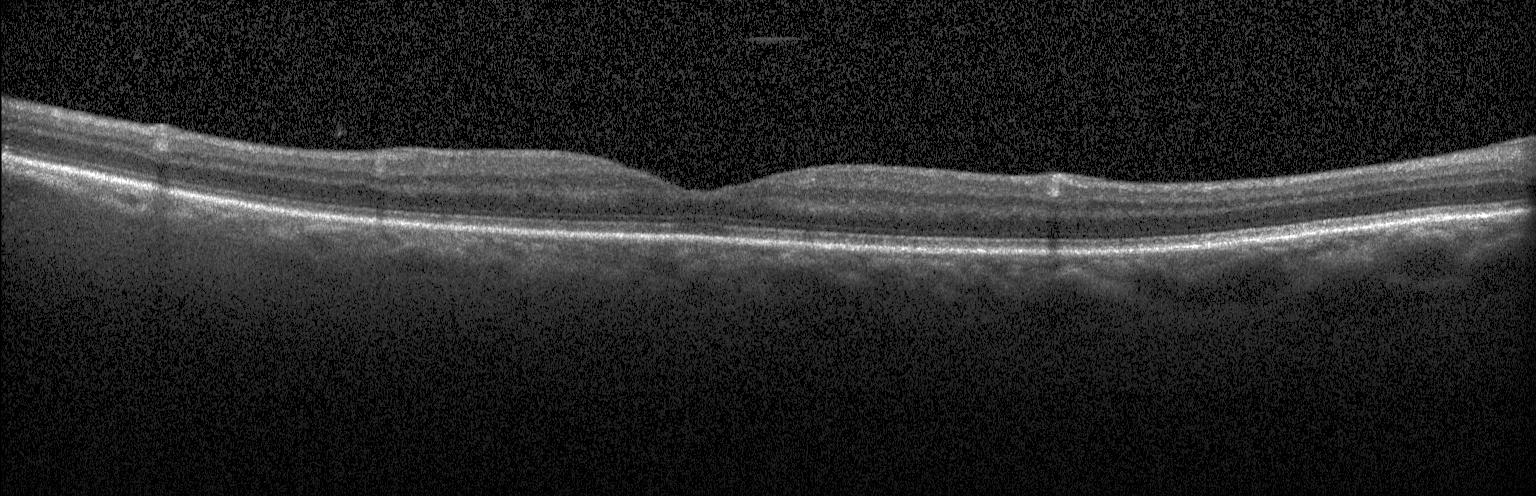 Horizontal scan through the fovea · SD-OCT · Heidelberg Spectralis · OCT B-scan.
Macular OCT: no choroidal neovascularization, no diabetic macular edema, and no drusen.